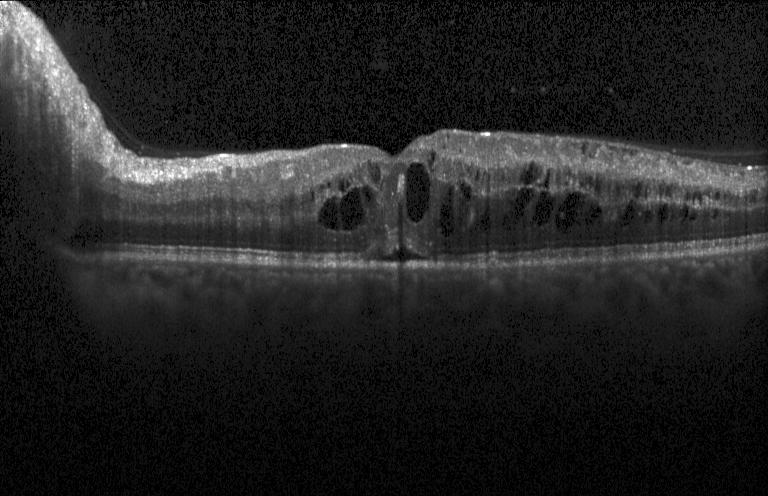 The scan shows diabetic macular edema (DME).